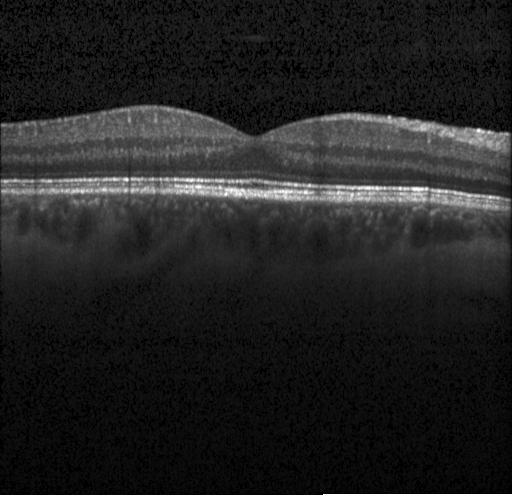

OCT line scan, instrument: Heidelberg Spectralis, SD-OCT. Impression: neither choroidal neovascularization, diabetic macular edema, nor drusen.